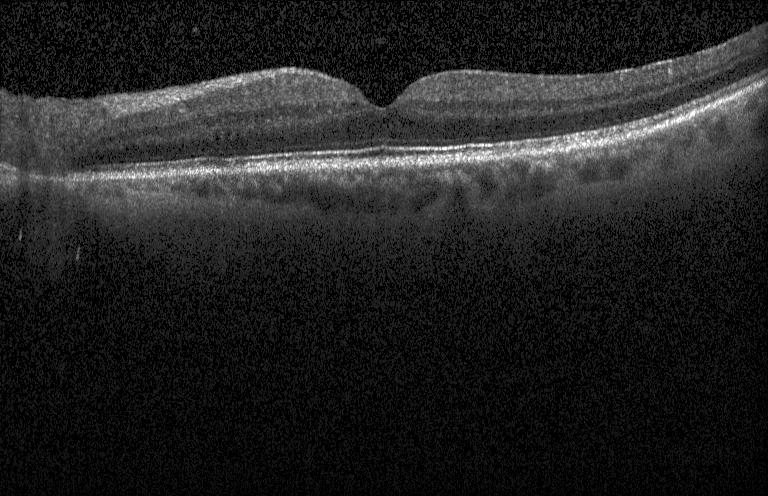

Retinal OCT cross-section, spectral-domain optical coherence tomography, Heidelberg Spectralis OCT system, horizontal scan through the fovea — The scan shows no evidence of CNV, DME, or drusen.